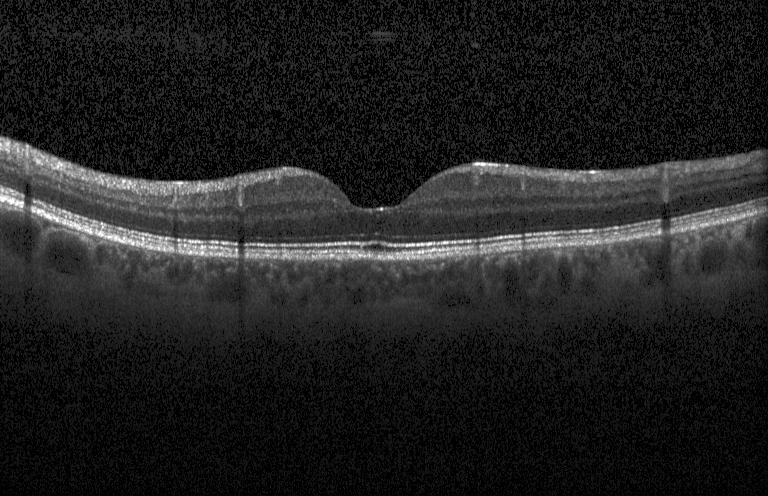
Optical coherence tomography B-scan; spectral-domain OCT; Heidelberg Spectralis. This B-scan demonstrates no choroidal neovascularization, no diabetic macular edema, and no drusen.